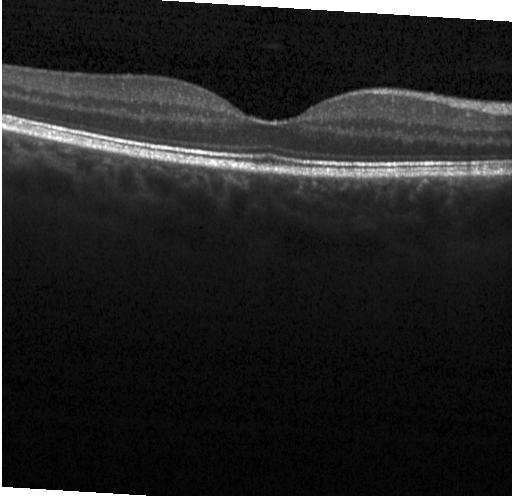
Spectral-domain OCT B-scan: neither CNV, DME, nor drusen.